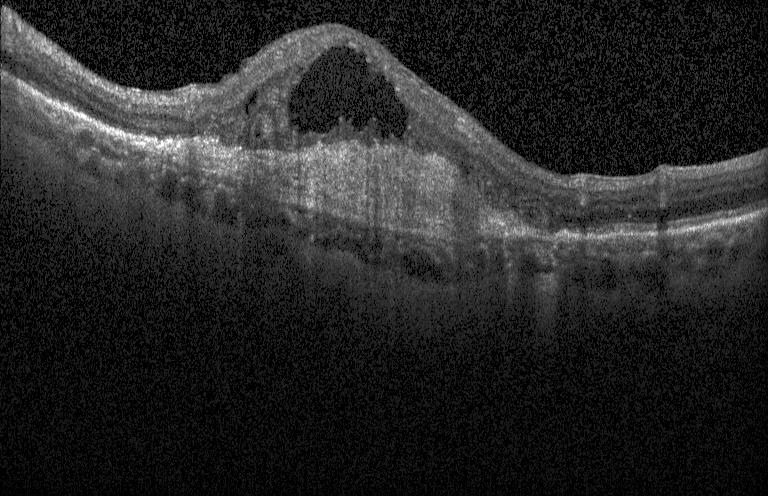 Impression: choroidal neovascularization (CNV).